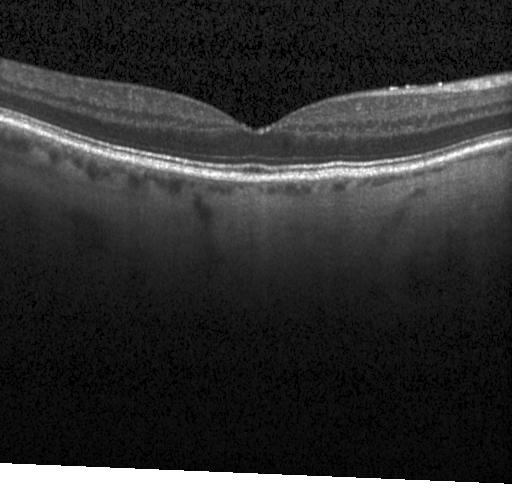

OCT line scan.
Diagnosis: neither CNV, DME, nor drusen.